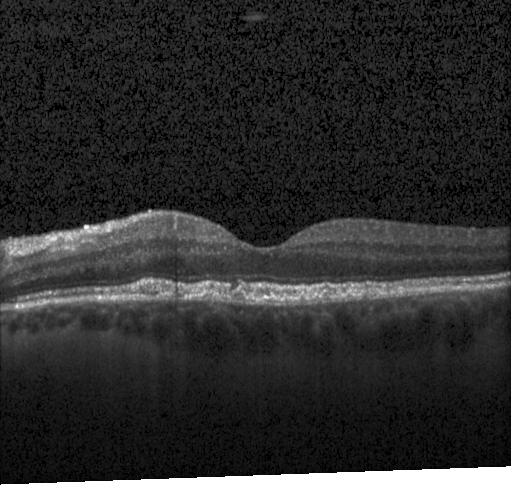
OCT line scan. Finding: sub-RPE drusenoid deposits.